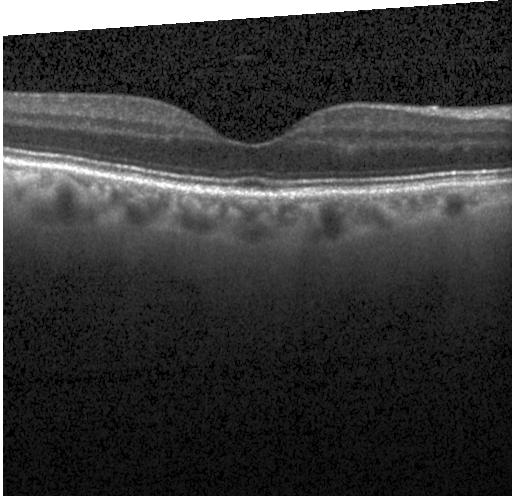 Retinal OCT B-scan
This B-scan demonstrates neither CNV, DME, nor drusen.